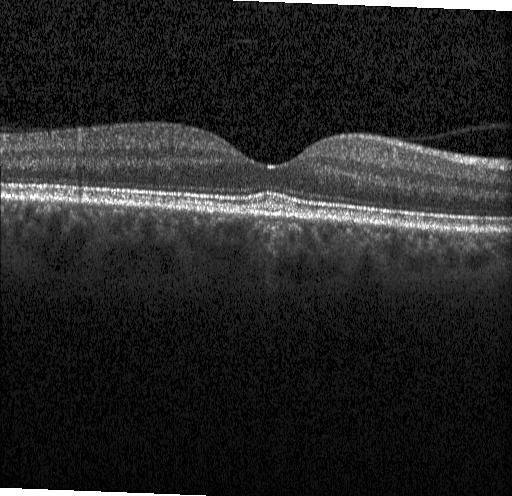
Impression: no CNV, no DME, and no drusen.